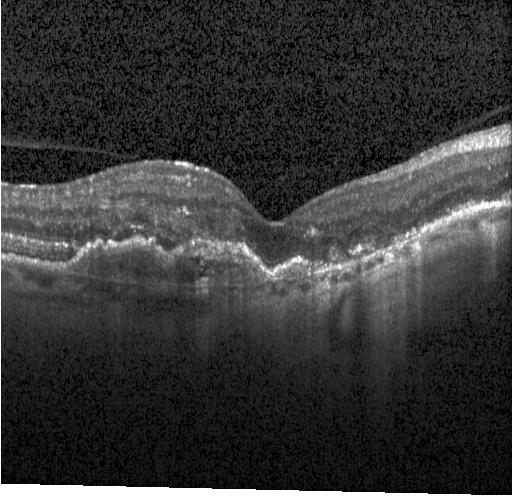

Heidelberg Spectralis OCT system · OCT B-scan — Diagnosis: a choroidal neovascular membrane.